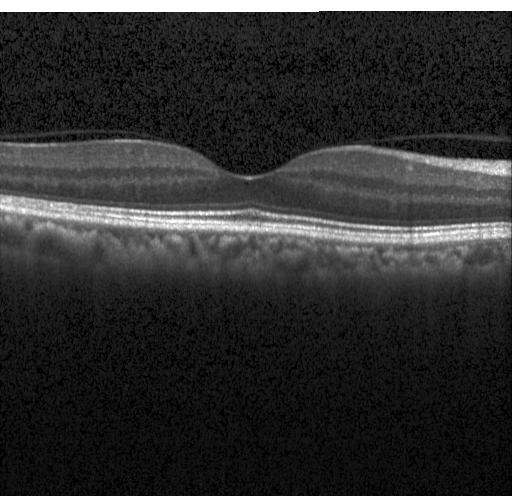
Retinal OCT B-scan · through the macula · Heidelberg Spectralis OCT system · SD-OCT.
Dx: no evidence of choroidal neovascularization, diabetic macular edema, or drusen.